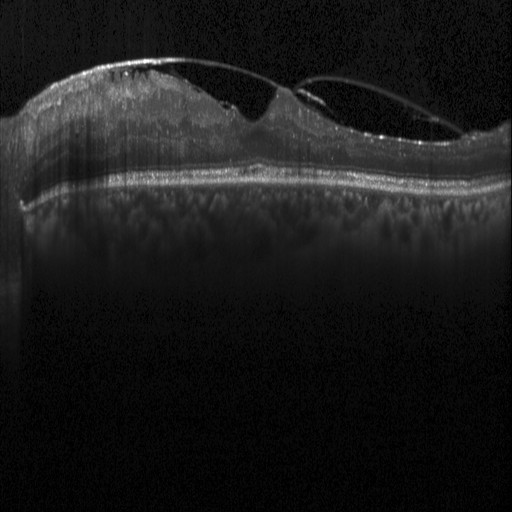
This B-scan demonstrates diabetic macular edema (DME).